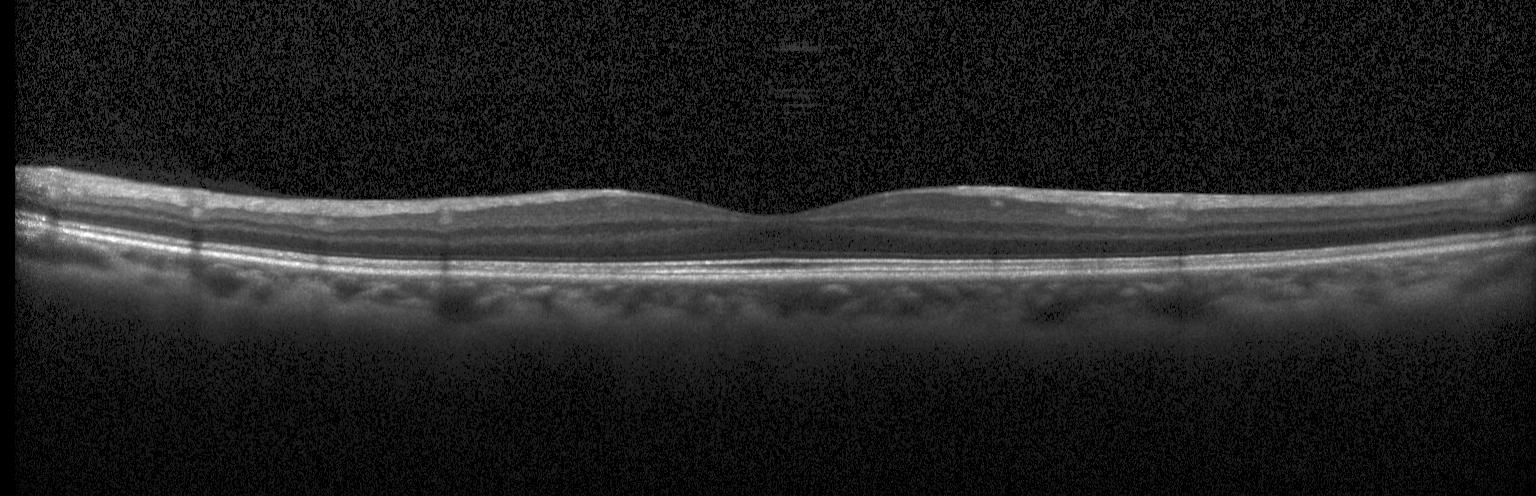 Retinal OCT cross-section.
Dx: neither CNV, DME, nor drusen.